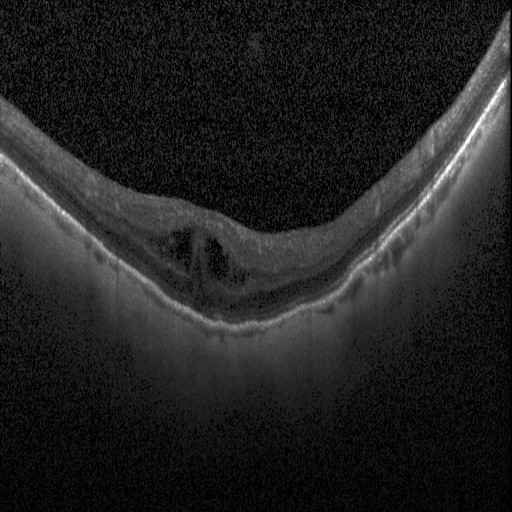
Centered on the fovea; optical coherence tomography scan; spectral-domain optical coherence tomography.
Macular OCT: DME.